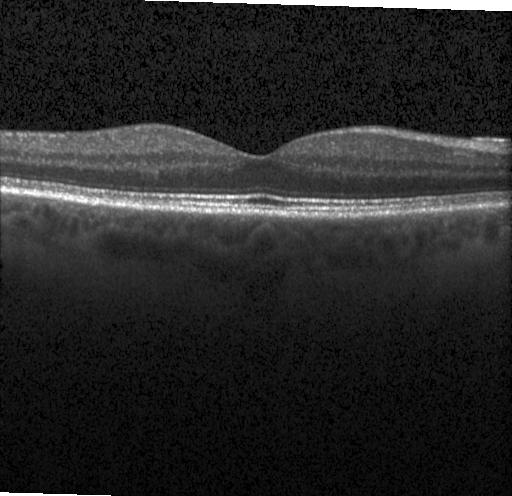

OCT B-scan, through the macula.
No choroidal neovascularization, diabetic macular edema, or drusen.